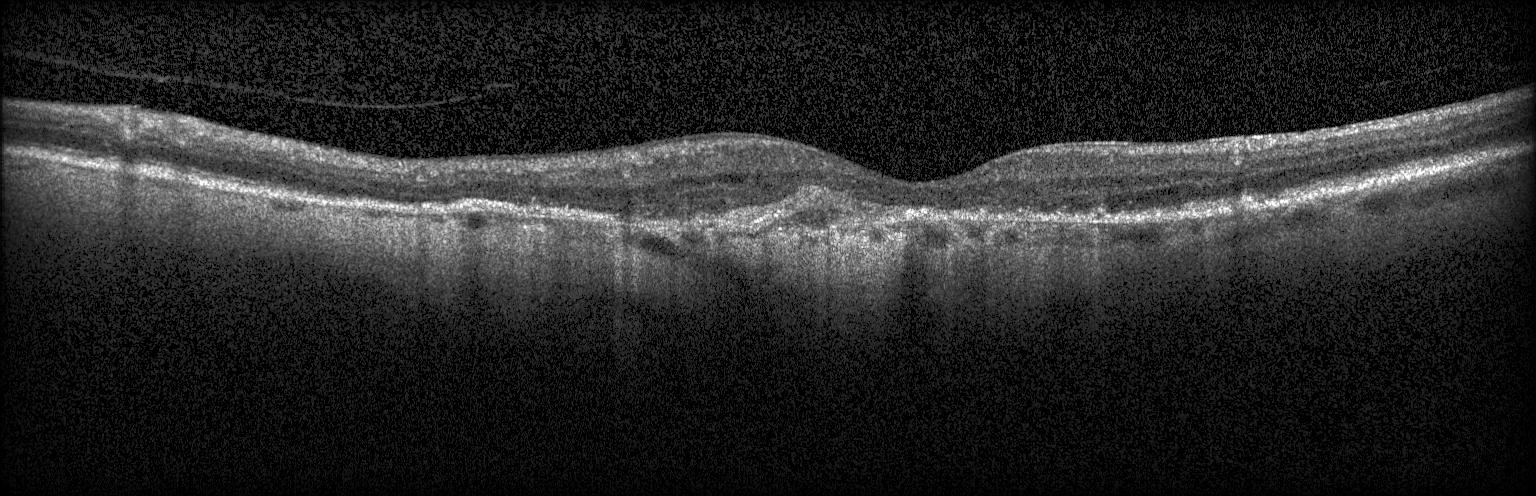
Macular OCT: a choroidal neovascular membrane.